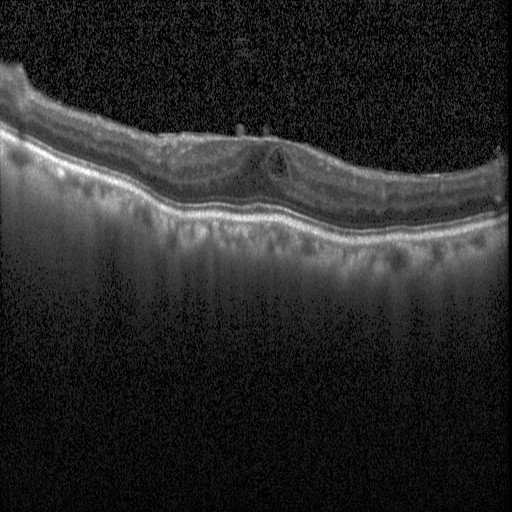 Impression: diabetic macular edema.